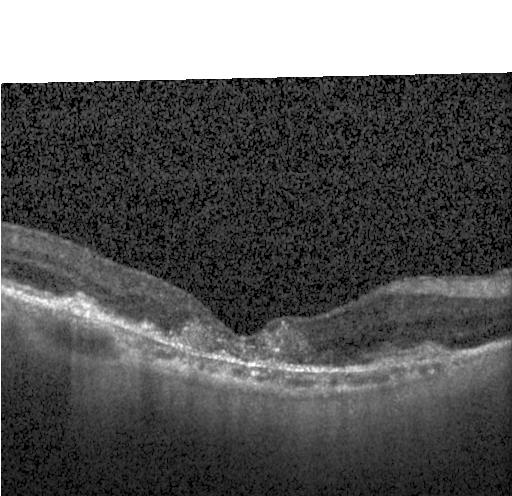 Spectral-domain optical coherence tomography. Instrument: Heidelberg Spectralis. Through the macula. Retinal OCT cross-section
The scan shows a choroidal neovascular membrane.